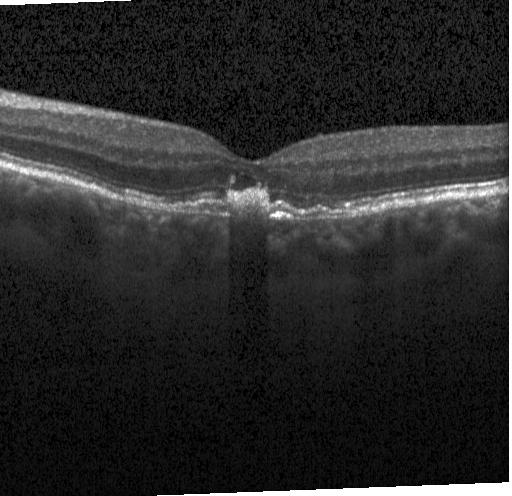 Fovea-centered · acquired on a Heidelberg Spectralis · OCT B-scan. Impression: choroidal neovascularization (CNV).